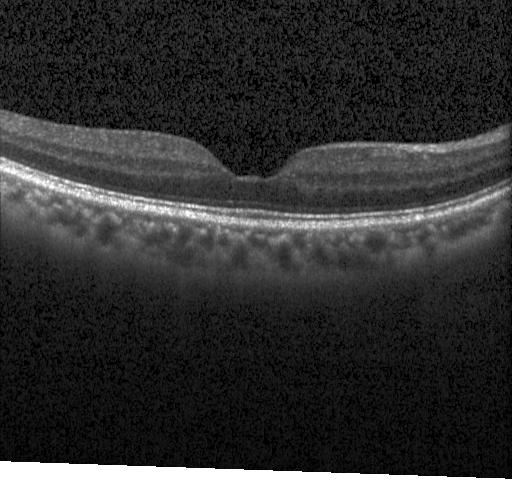
SD-OCT · optical coherence tomography scan · Heidelberg Spectralis OCT system — OCT finding: no choroidal neovascularization, diabetic macular edema, or drusen.